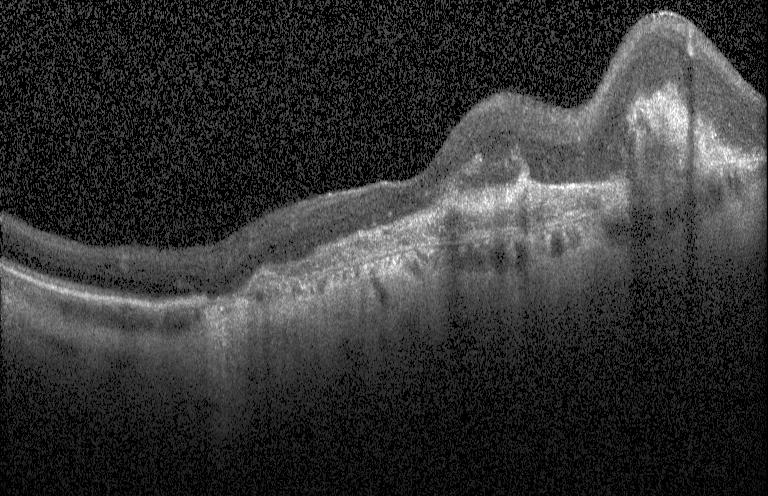
Choroidal neovascularization (CNV).